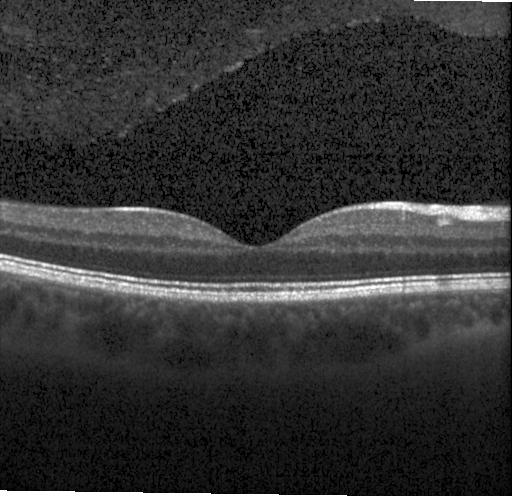 Acquired on a Heidelberg Spectralis. Horizontal scan through the fovea. Spectral-domain optical coherence tomography. Retinal OCT B-scan.
Diagnosis: neither choroidal neovascularization, diabetic macular edema, nor drusen.